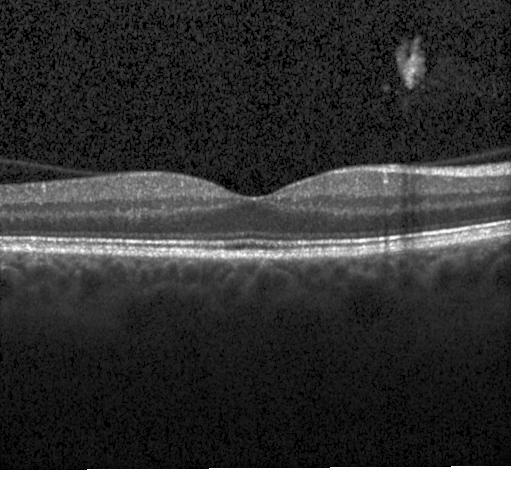
Macular OCT: no evidence of choroidal neovascularization, diabetic macular edema, or drusen.